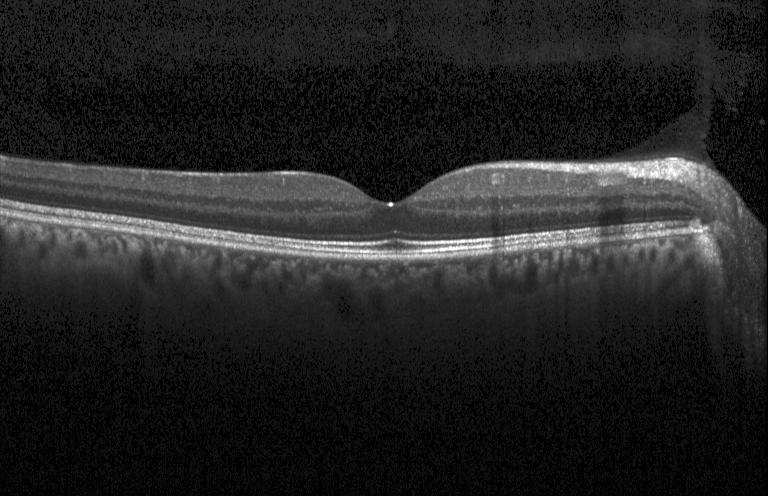
Retinal OCT cross-section, spectral-domain optical coherence tomography, instrument: Heidelberg Spectralis
Macular OCT: no CNV, no DME, and no drusen.